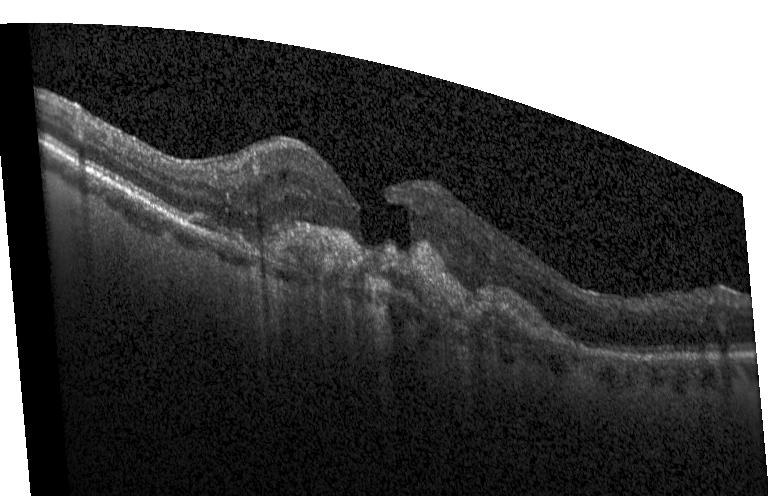

OCT scan showing a choroidal neovascular membrane.